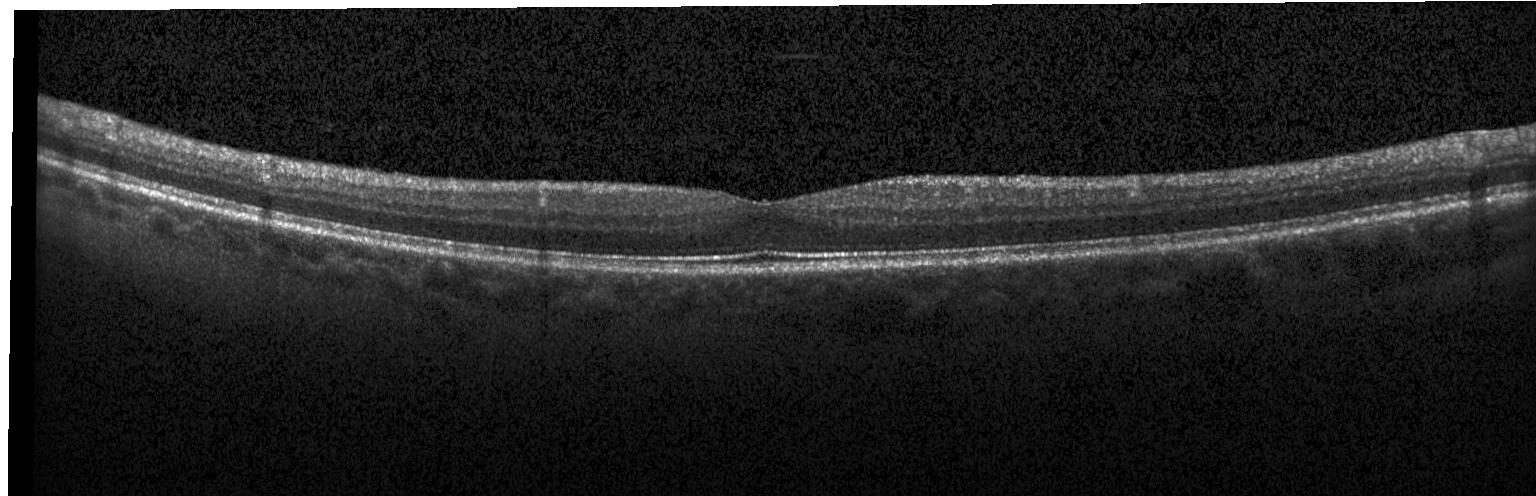
Spectral-domain OCT · OCT B-scan · acquired on a Heidelberg Spectralis. Impression: no evidence of choroidal neovascularization, diabetic macular edema, or drusen.